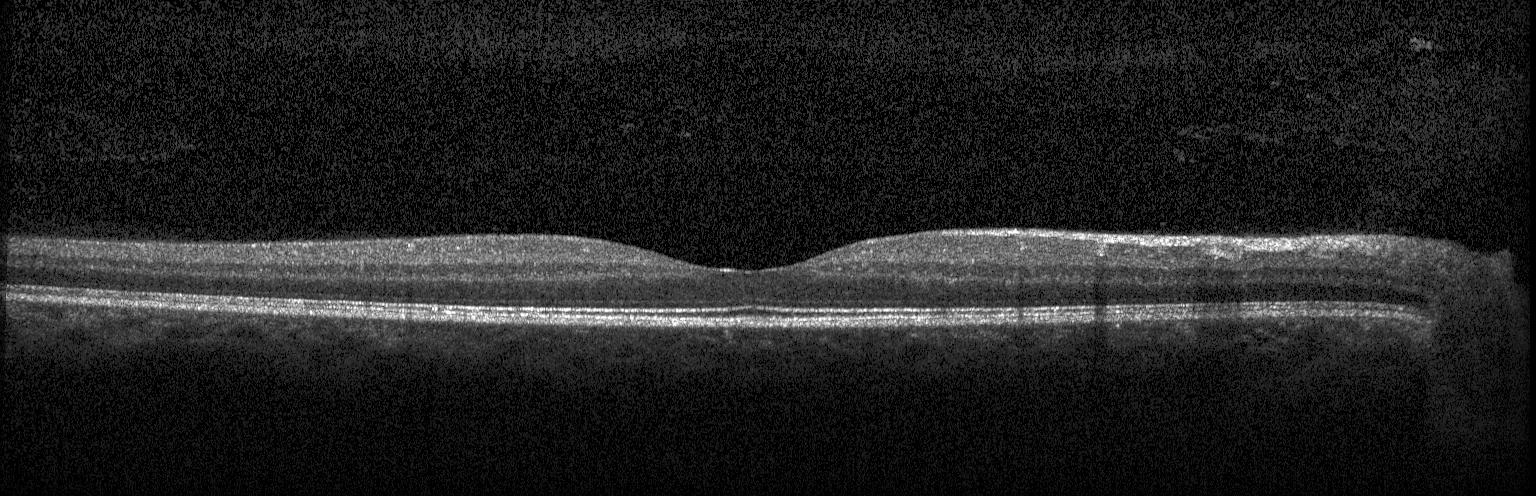 Assessment: no evidence of choroidal neovascularization, diabetic macular edema, or drusen.